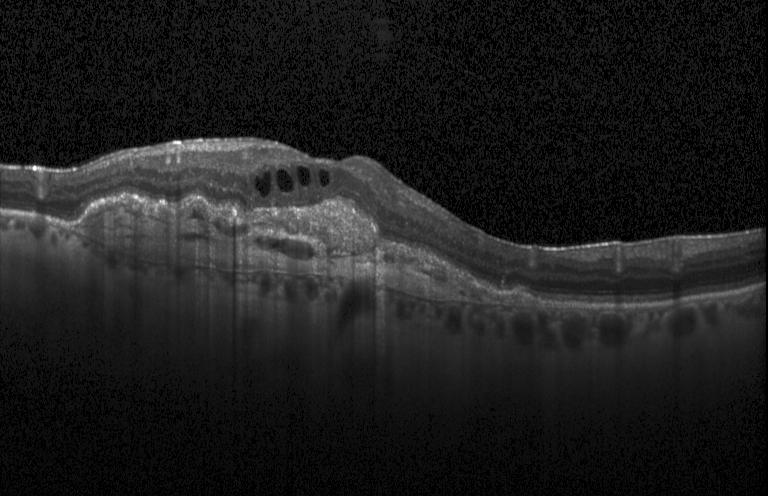
Retinal OCT cross-section. Finding: choroidal neovascularization.